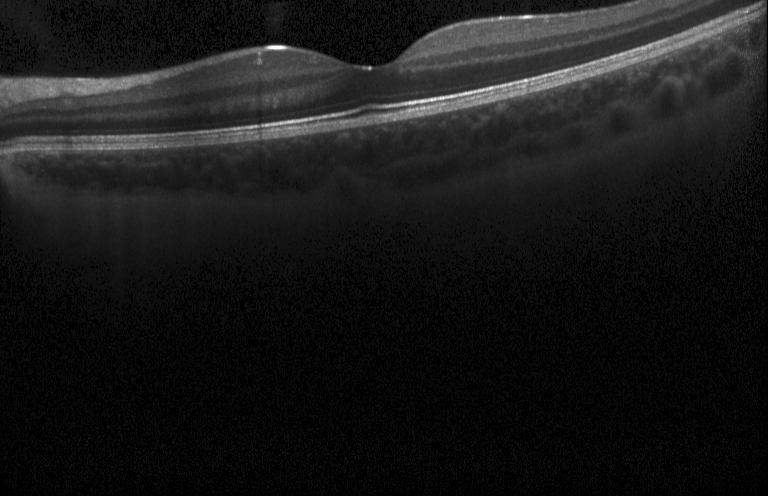 Spectral-domain OCT B-scan: no evidence of choroidal neovascularization, diabetic macular edema, or drusen.